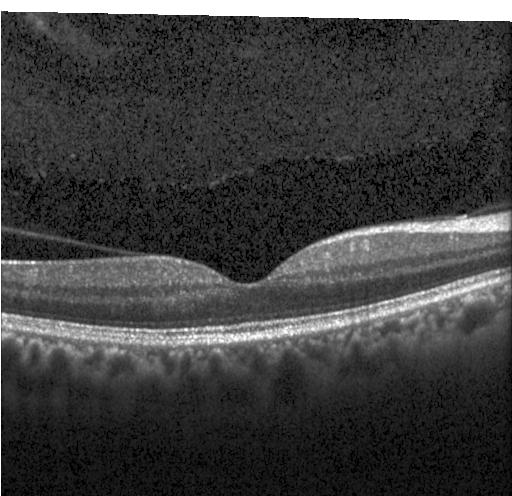

Through the macula. OCT B-scan. This B-scan demonstrates no choroidal neovascularization, diabetic macular edema, or drusen.